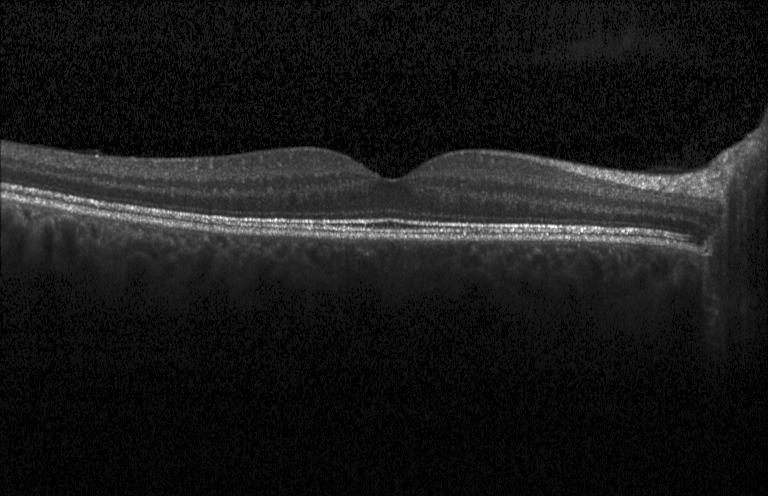

Centered on the fovea. Spectral-domain optical coherence tomography. Instrument: Heidelberg Spectralis. Retinal OCT B-scan.
This B-scan demonstrates no choroidal neovascularization, diabetic macular edema, or drusen.